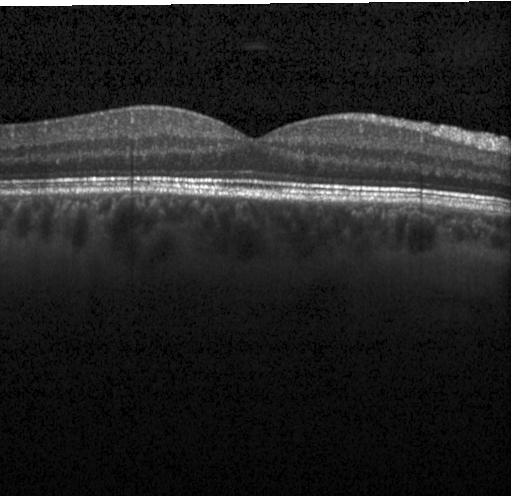 Retinal OCT cross-section showing no choroidal neovascularization, diabetic macular edema, or drusen.